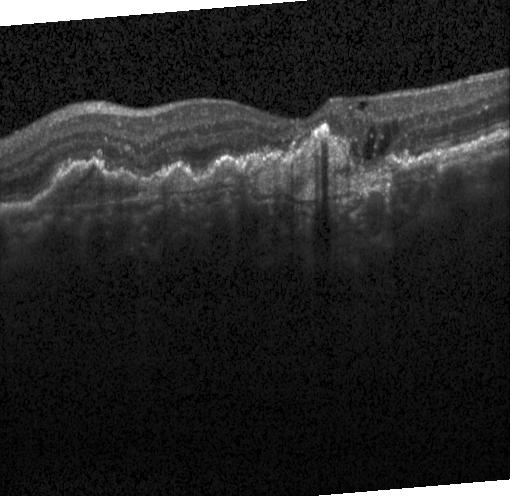

Retinal OCT B-scan · acquired on a Heidelberg Spectralis · spectral-domain optical coherence tomography — Finding: choroidal neovascularization.